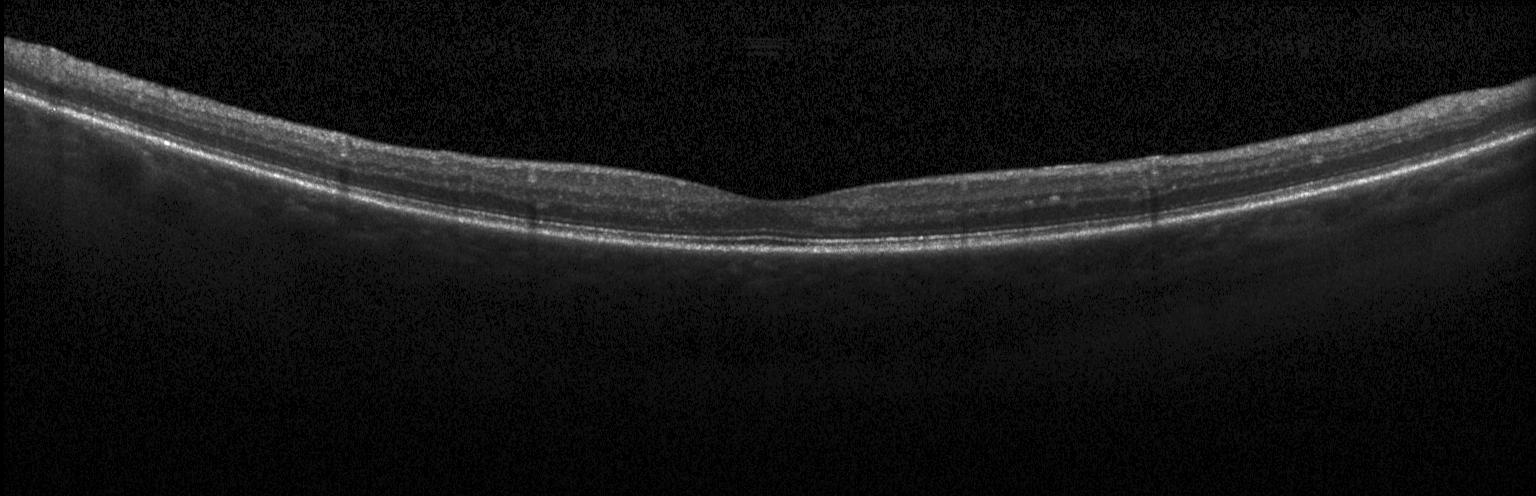 Retinal OCT cross-section. Acquired on a Heidelberg Spectralis. Macular scan. Spectral-domain OCT. Finding: no choroidal neovascularization, no diabetic macular edema, and no drusen.